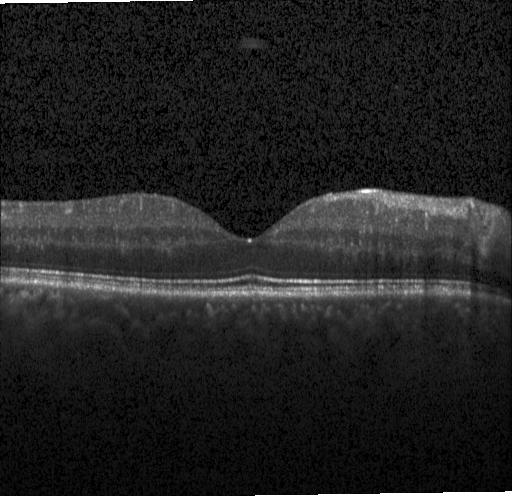 OCT line scan · macular scan · spectral-domain optical coherence tomography · instrument: Heidelberg Spectralis
Dx: no evidence of choroidal neovascularization, diabetic macular edema, or drusen.